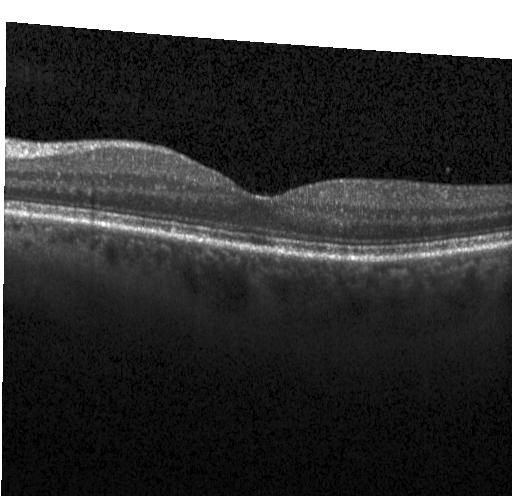

OCT line scan. Diagnosis: no choroidal neovascularization, diabetic macular edema, or drusen.